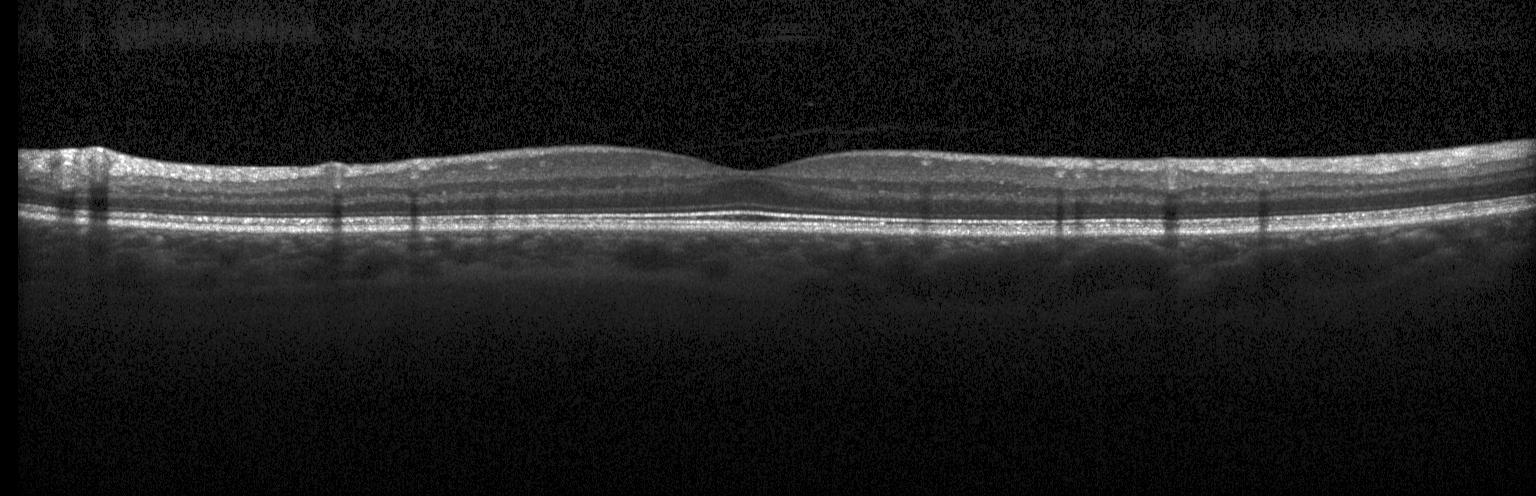

Dx: no choroidal neovascularization, no diabetic macular edema, and no drusen.